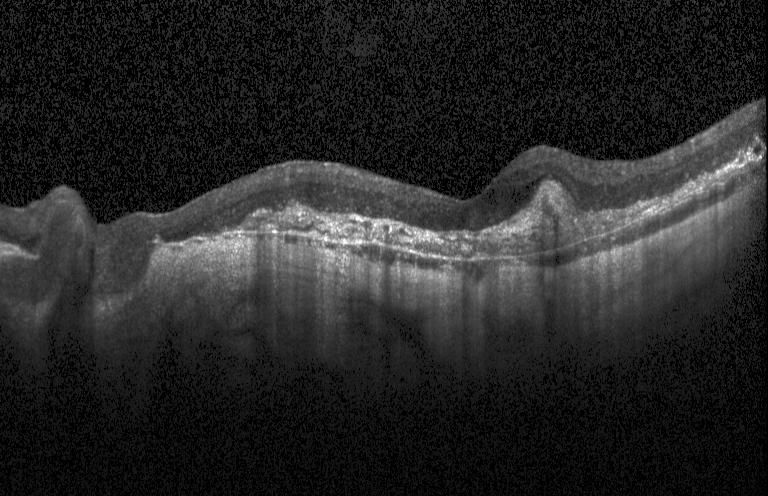

Impression: a choroidal neovascular membrane.